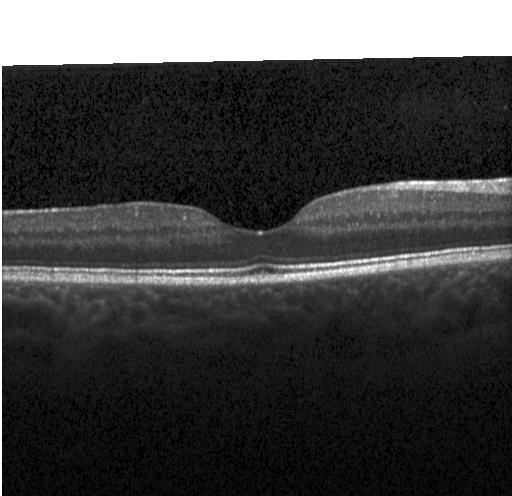

Macular OCT: neither choroidal neovascularization, diabetic macular edema, nor drusen.